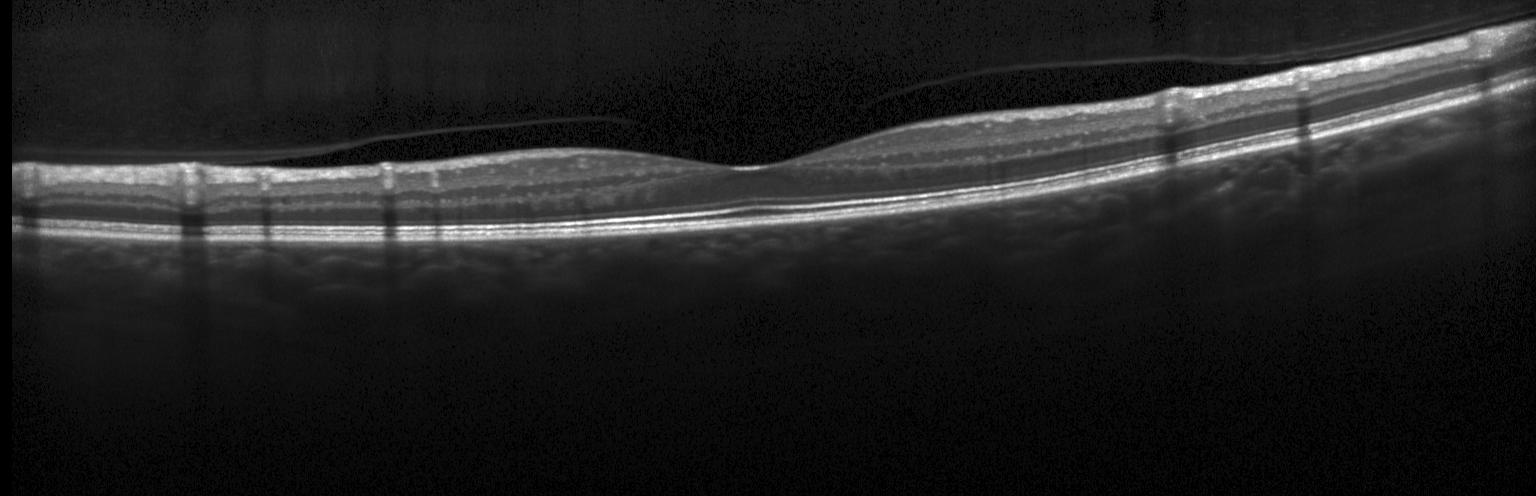 Spectral-domain OCT · retinal OCT cross-section. Assessment: no choroidal neovascularization, no diabetic macular edema, and no drusen.